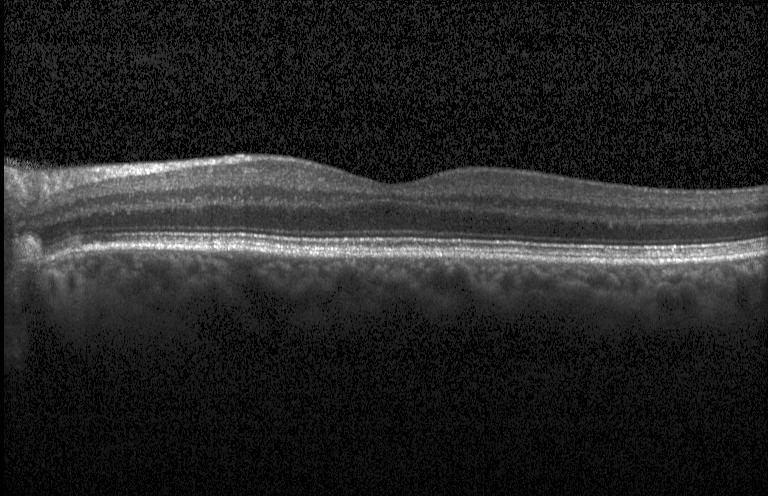

Heidelberg Spectralis, spectral-domain OCT, optical coherence tomography scan
The scan shows no choroidal neovascularization, no diabetic macular edema, and no drusen.